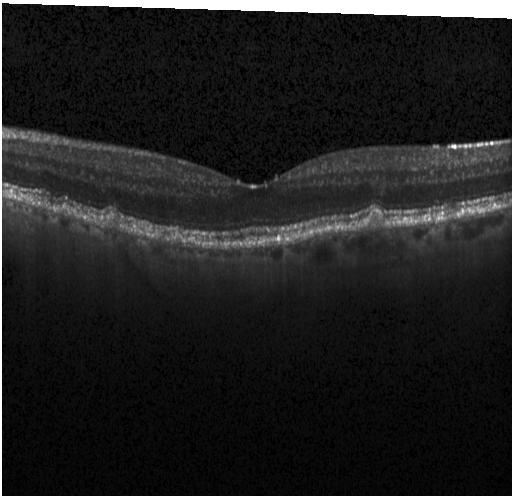
Dx: multiple drusen.